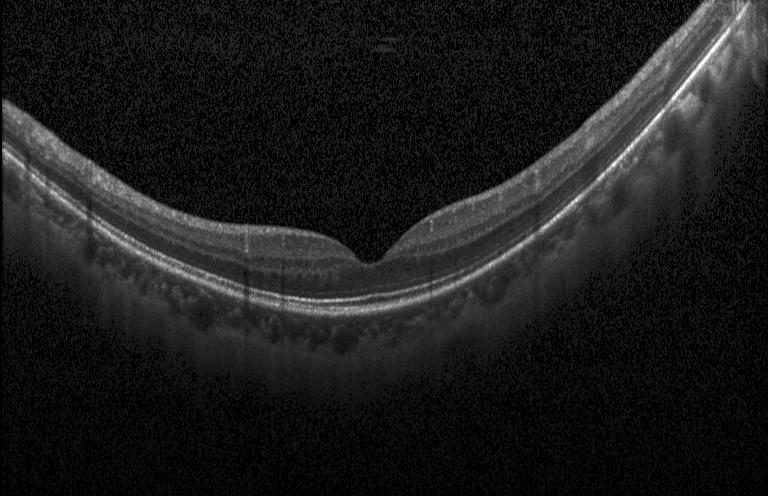
OCT B-scan.
Macular OCT: no choroidal neovascularization, no diabetic macular edema, and no drusen.